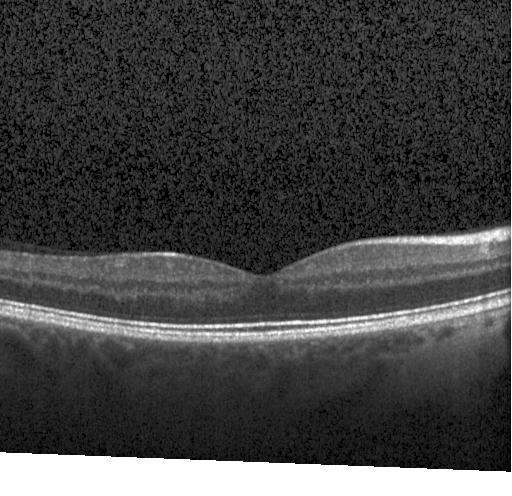
Horizontal scan through the fovea · spectral-domain OCT · instrument: Heidelberg Spectralis · retinal OCT cross-section — Diagnosis: no evidence of CNV, DME, or drusen.